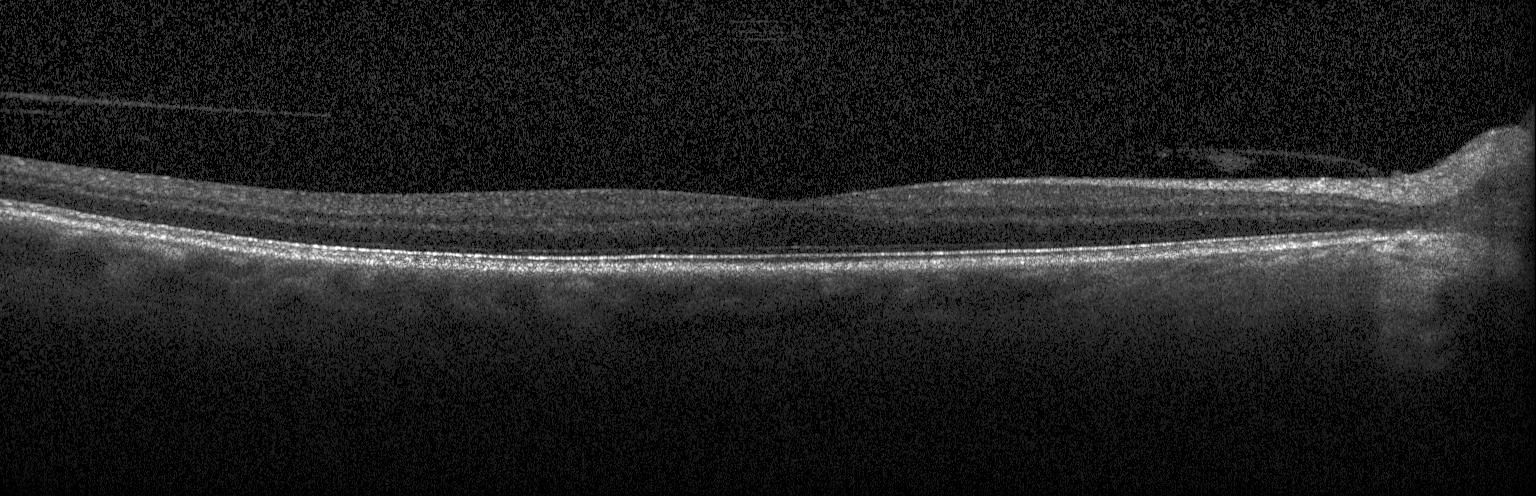
Fovea-centered, Heidelberg Spectralis, OCT line scan, SD-OCT — Impression: no evidence of choroidal neovascularization, diabetic macular edema, or drusen.